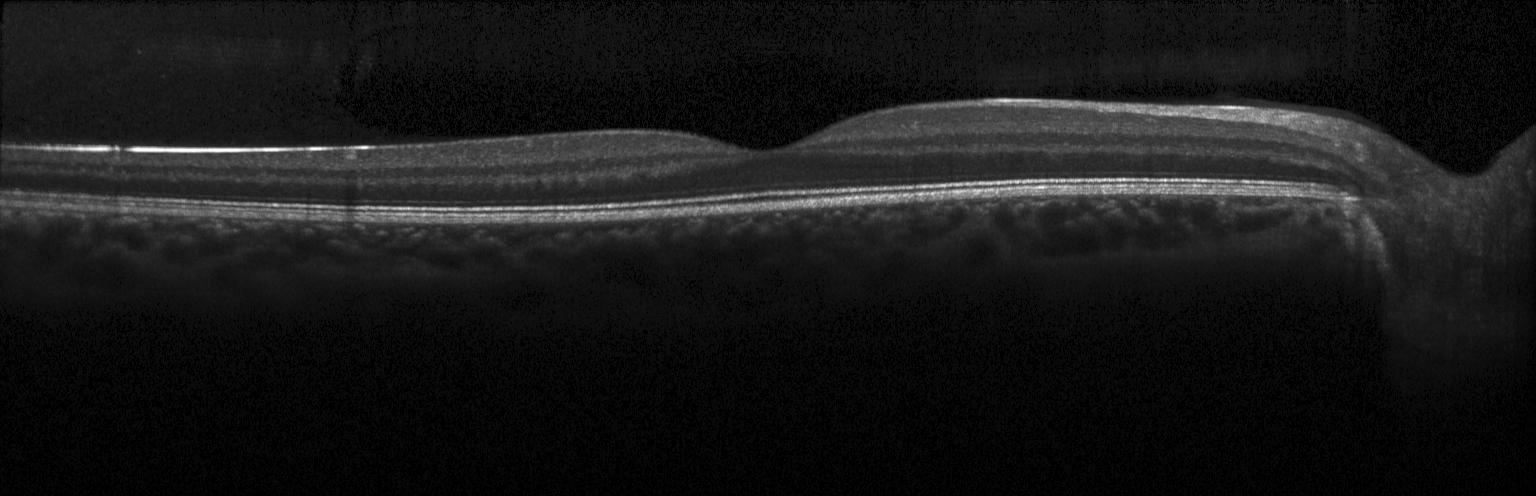

Retinal OCT cross-section showing no choroidal neovascularization, diabetic macular edema, or drusen.